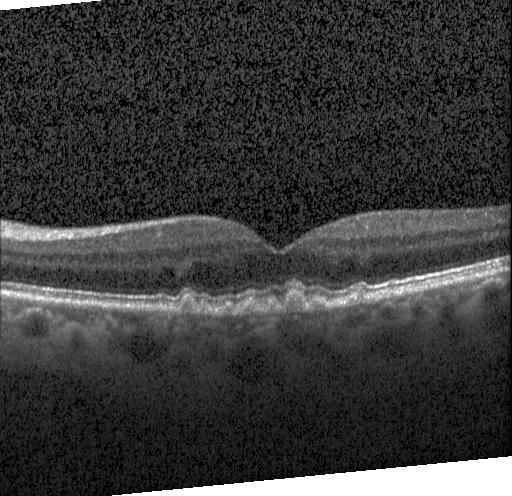
OCT finding: multiple drusen.